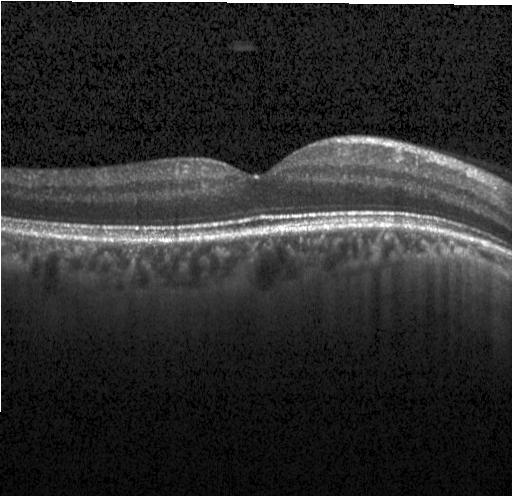 OCT B-scan. Dx: no CNV, no DME, and no drusen.